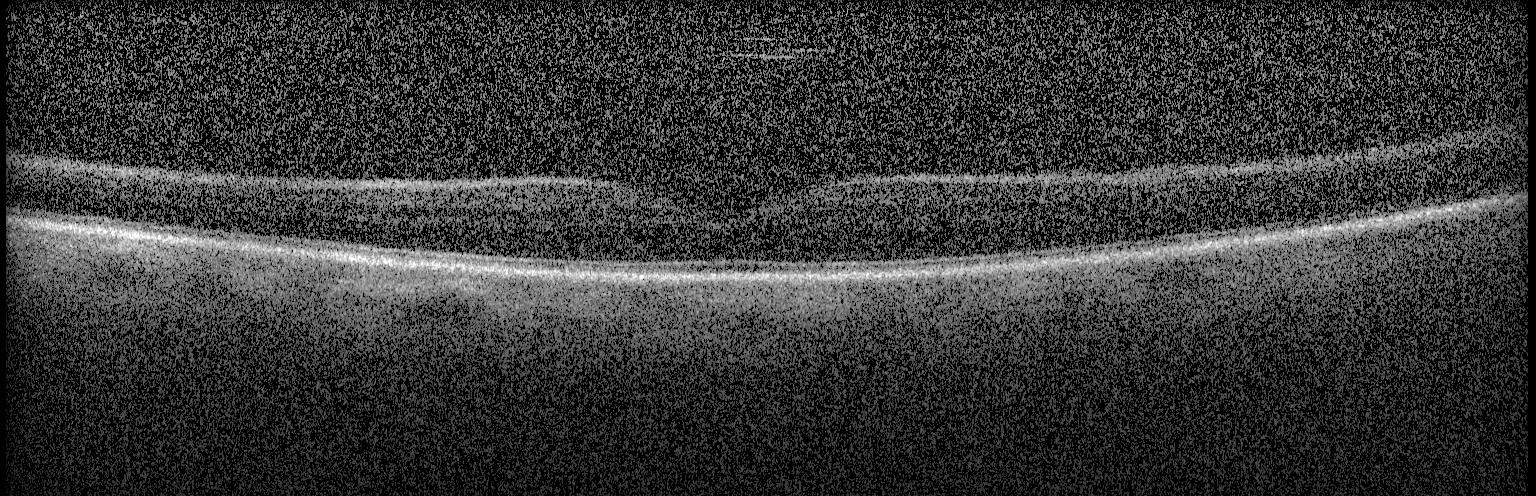
SD-OCT, through the macula, OCT line scan. Impression: neither choroidal neovascularization, diabetic macular edema, nor drusen.